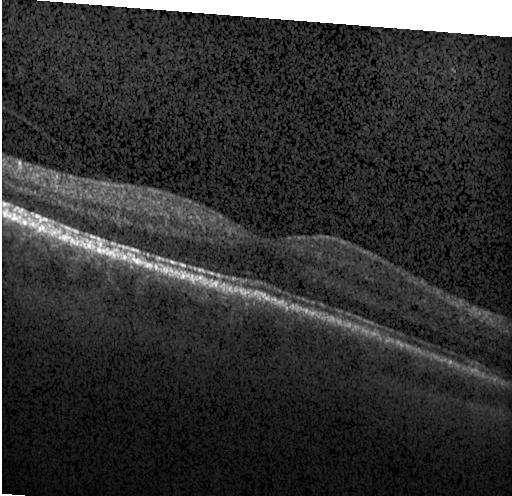 Optical coherence tomography B-scan. The scan shows neither choroidal neovascularization, diabetic macular edema, nor drusen.